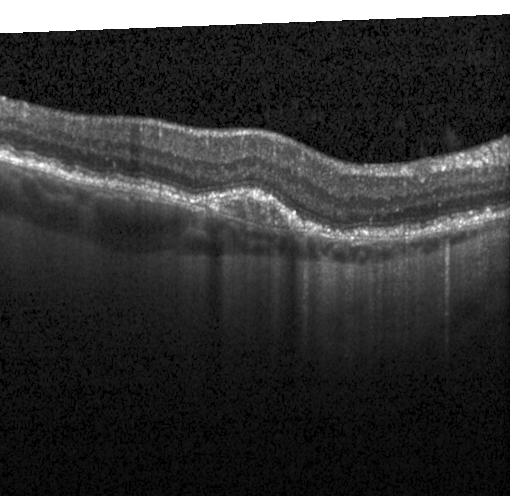
Heidelberg Spectralis, macular scan, OCT line scan
Macular OCT: CNV.